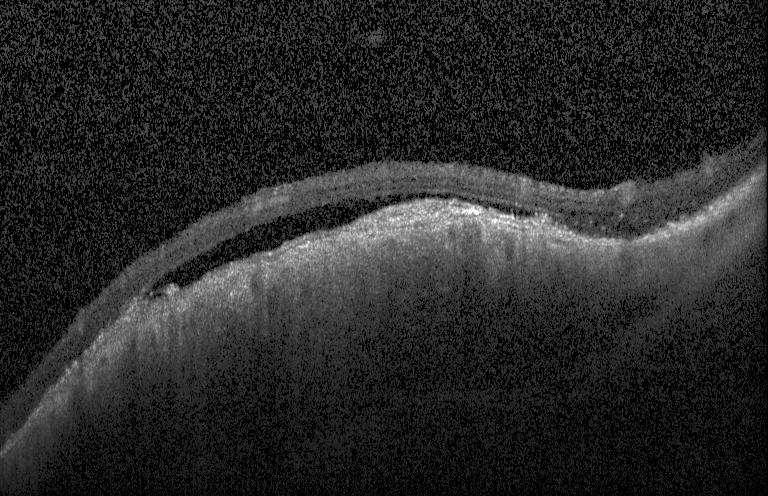
Retinal OCT cross-section showing CNV.